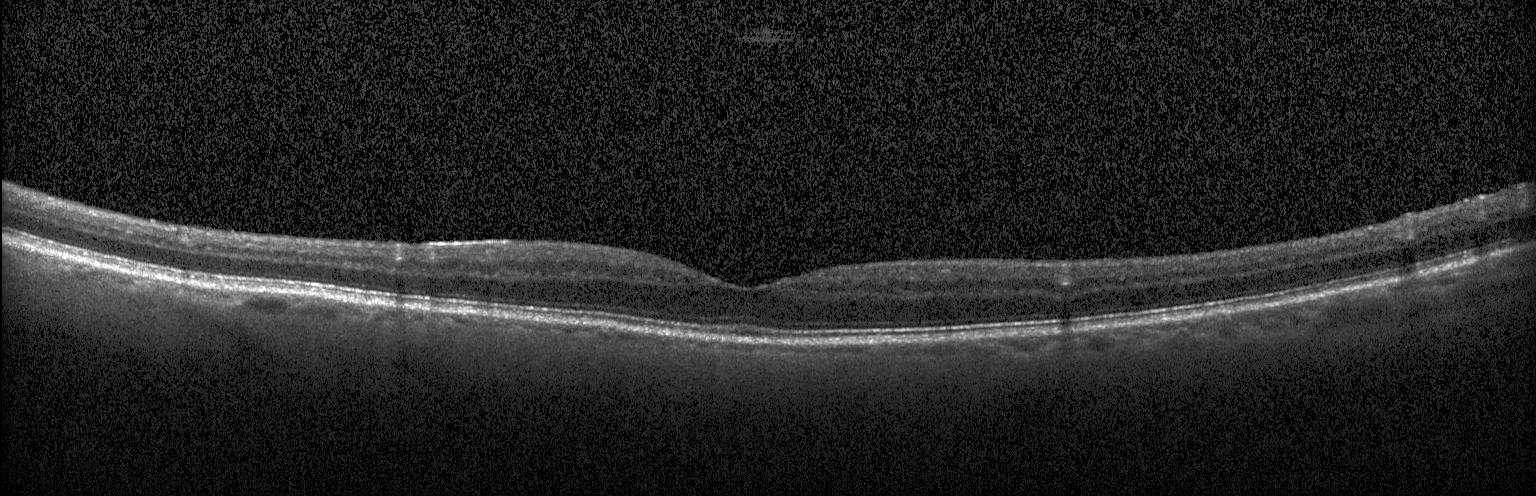 Dx: neither CNV, DME, nor drusen.